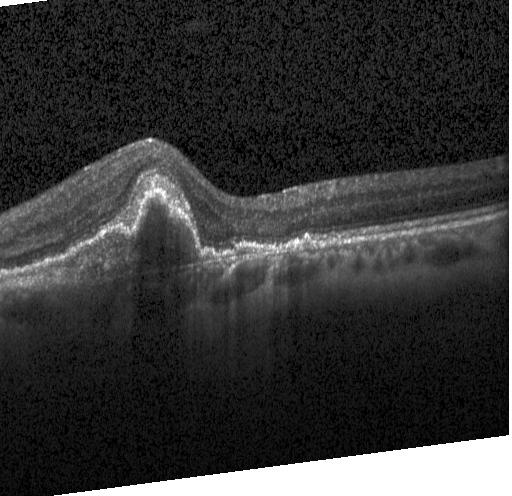 Macular OCT demonstrating CNV.